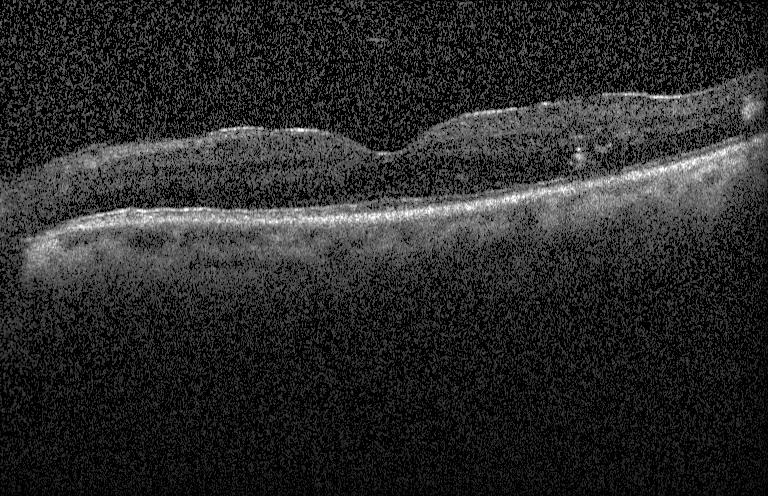
Optical coherence tomography scan. Centered on the fovea. Heidelberg Spectralis OCT system.
Macular OCT: no choroidal neovascularization, no diabetic macular edema, and no drusen.